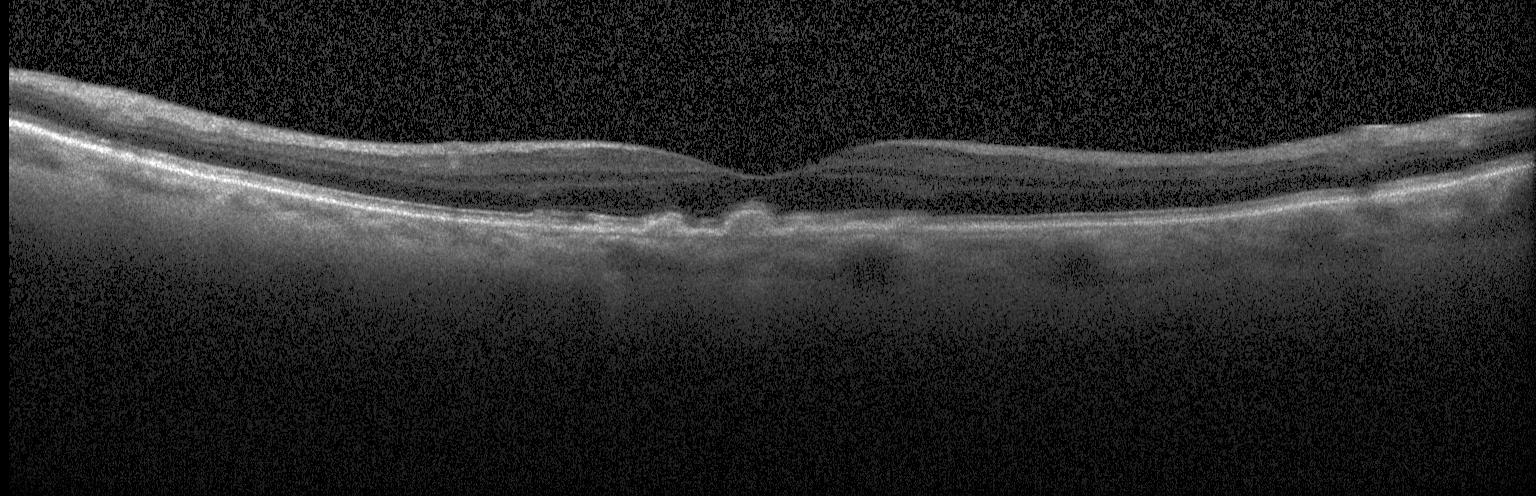 OCT line scan · instrument: Heidelberg Spectralis · macular scan · spectral-domain optical coherence tomography.
Assessment: multiple drusen.